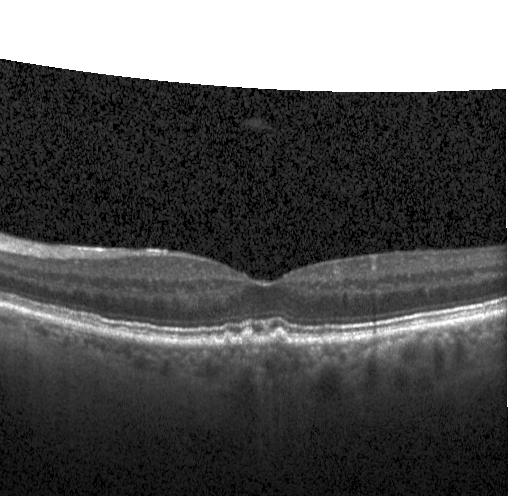 The scan shows drusen.